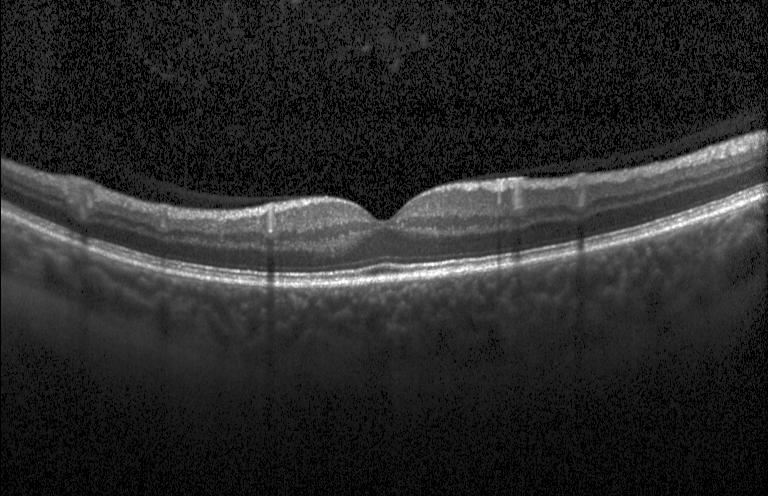 Retinal OCT cross-section, Heidelberg Spectralis — Diagnosis: no evidence of CNV, DME, or drusen.